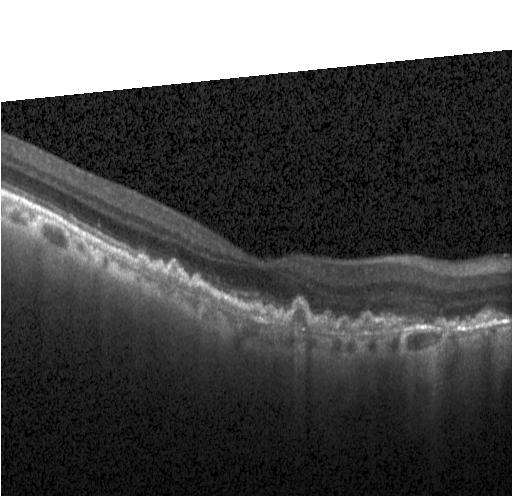 Optical coherence tomography B-scan, instrument: Heidelberg Spectralis, SD-OCT, horizontal scan through the fovea — Impression: a choroidal neovascular membrane.